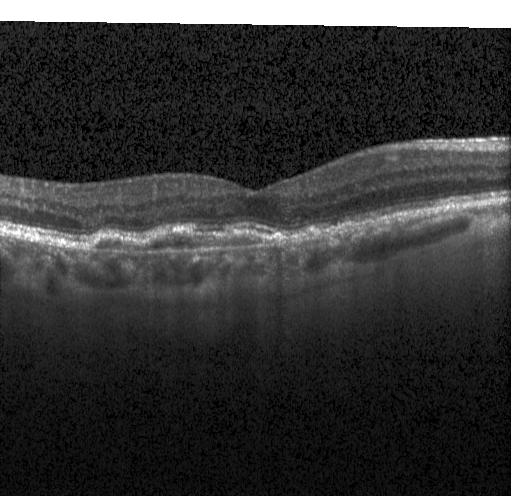

Dx: CNV.